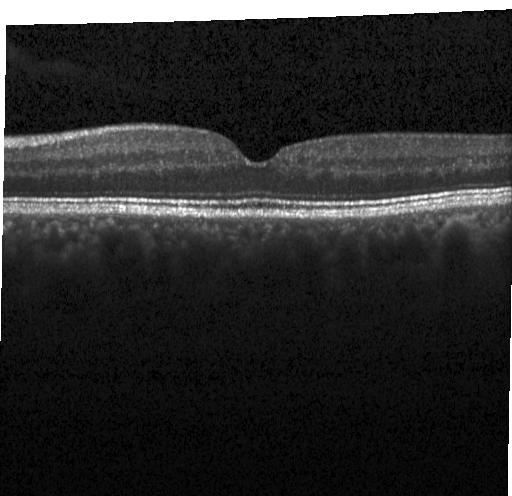 Heidelberg Spectralis; retinal OCT cross-section.
This B-scan demonstrates neither CNV, DME, nor drusen.